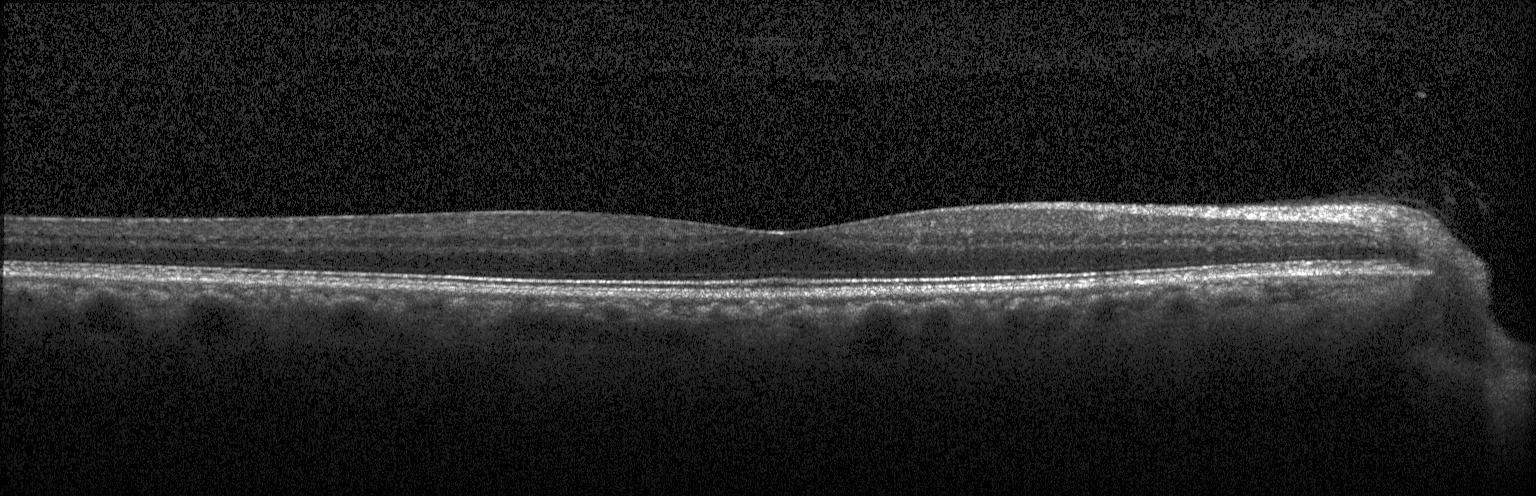

Impression: no choroidal neovascularization, no diabetic macular edema, and no drusen.